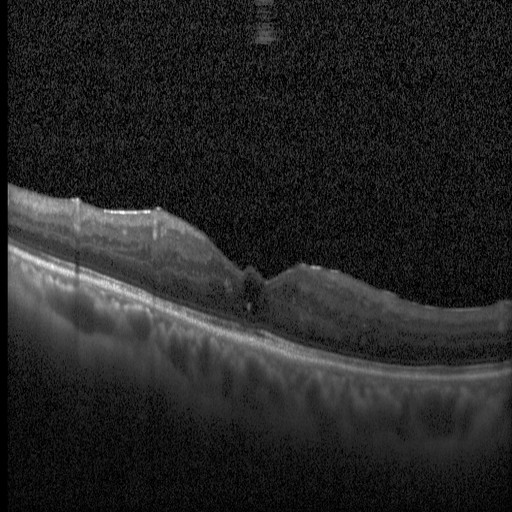 Optical coherence tomography B-scan. Acquired on a Heidelberg Spectralis. Spectral-domain optical coherence tomography. Horizontal scan through the fovea — This B-scan demonstrates diabetic macular edema.